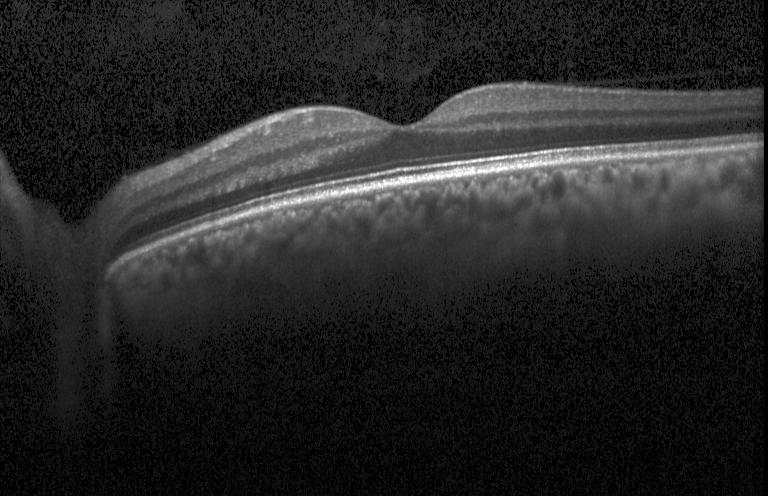
Finding: no choroidal neovascularization, diabetic macular edema, or drusen.